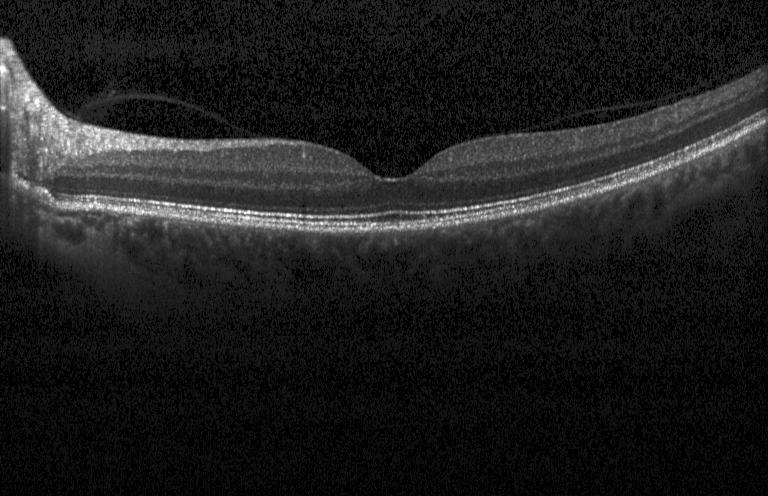 Fovea-centered; spectral-domain OCT; retinal OCT B-scan.
Macular OCT: no CNV, DME, or drusen.